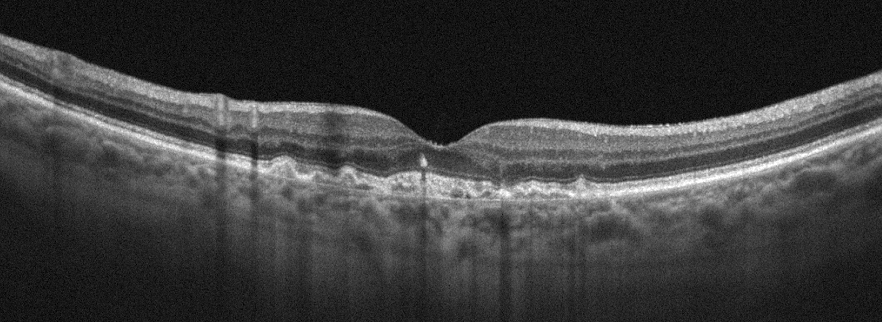

Right eye. Retinal OCT cross-section. Through the macula — Dx: age-related macular degeneration (AMD).